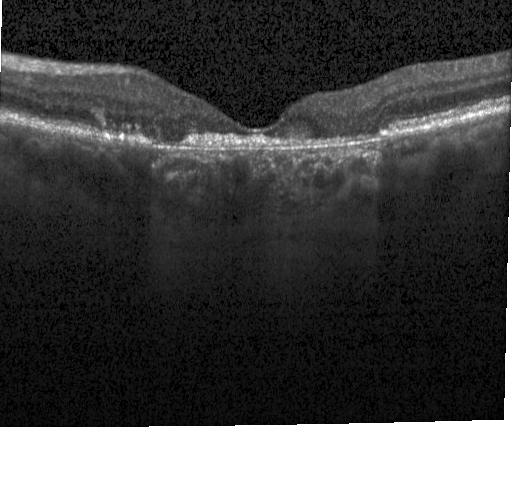

Acquired on a Heidelberg Spectralis, fovea-centered, optical coherence tomography scan.
OCT finding: CNV.